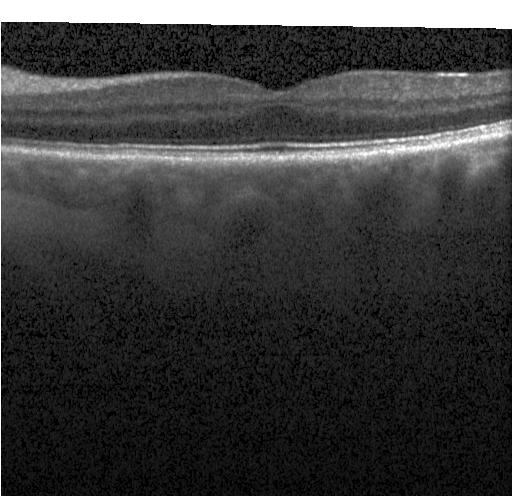

OCT scan showing no evidence of CNV, DME, or drusen.